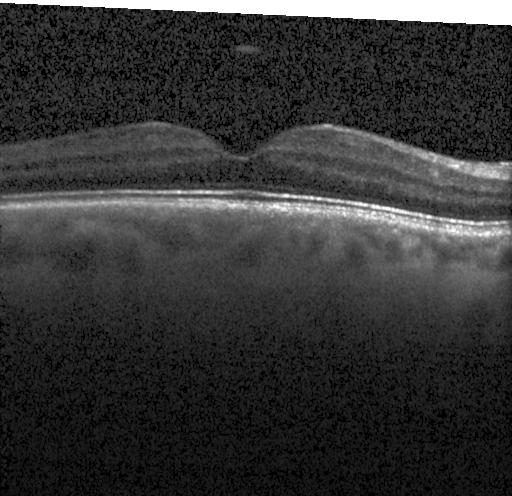 OCT line scan, Heidelberg Spectralis OCT system. Finding: no evidence of CNV, DME, or drusen.